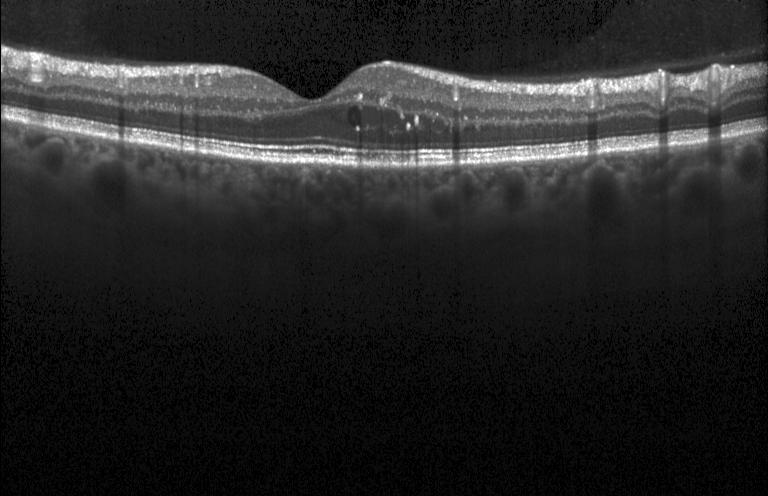
Instrument: Heidelberg Spectralis; through the macula; SD-OCT; OCT line scan
Impression: DME.